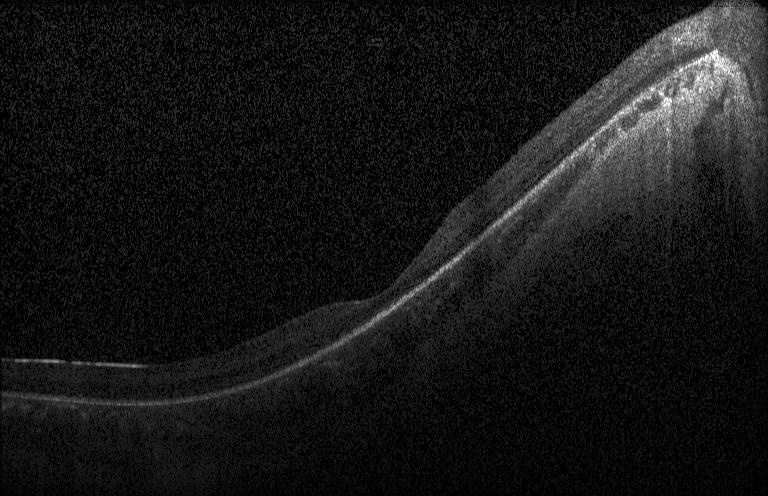
Spectral-domain optical coherence tomography · instrument: Heidelberg Spectralis · OCT B-scan · macular scan
No choroidal neovascularization, no diabetic macular edema, and no drusen.